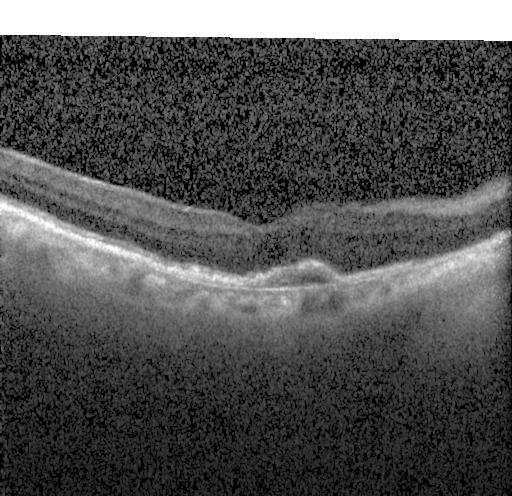 SD-OCT; retinal OCT cross-section.
Finding: a choroidal neovascular membrane.